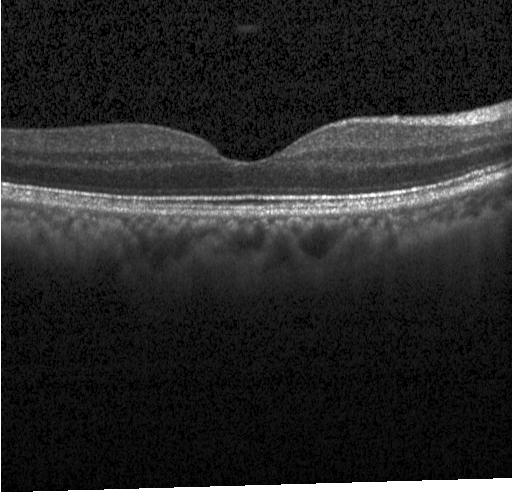 OCT scan showing no choroidal neovascularization, no diabetic macular edema, and no drusen.